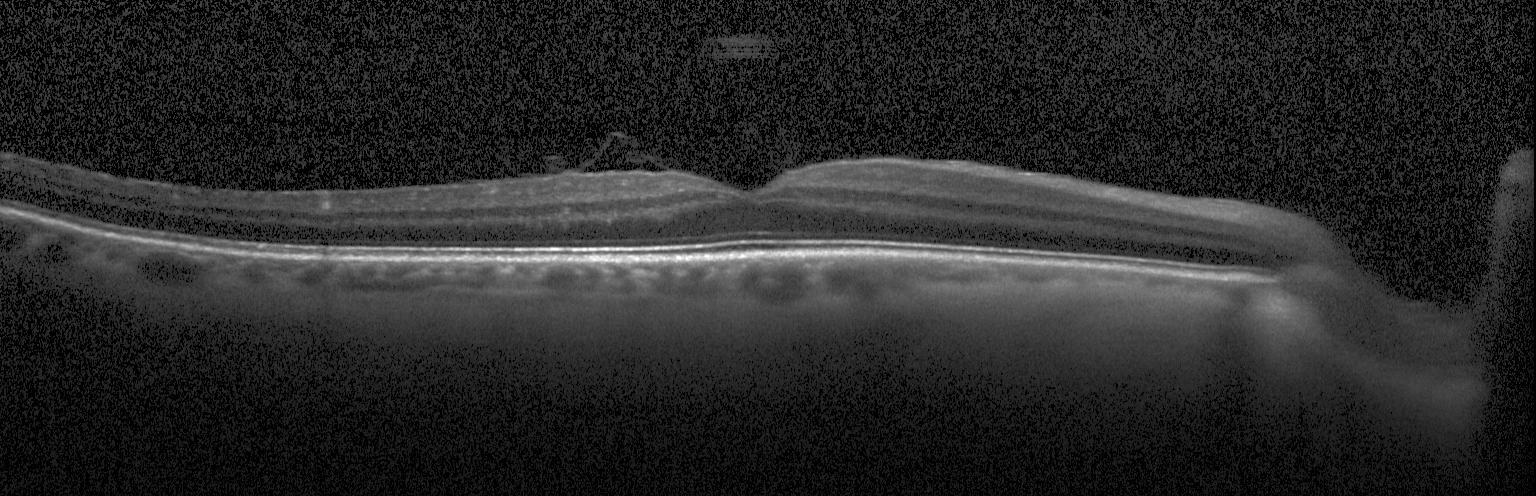

Optical coherence tomography B-scan. Heidelberg Spectralis OCT system. Macular scan. Spectral-domain OCT.
No choroidal neovascularization, no diabetic macular edema, and no drusen.